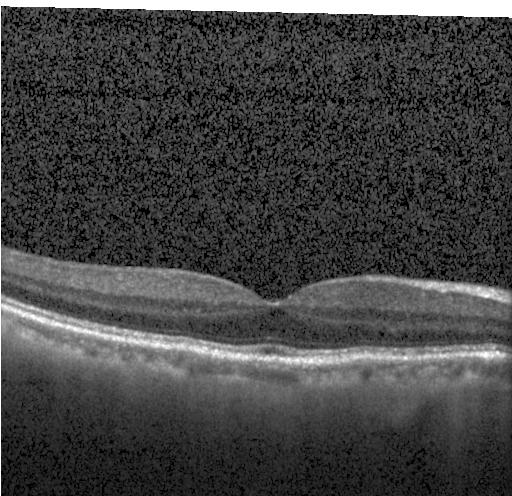
SD-OCT. Heidelberg Spectralis. Optical coherence tomography B-scan
Assessment: neither CNV, DME, nor drusen.